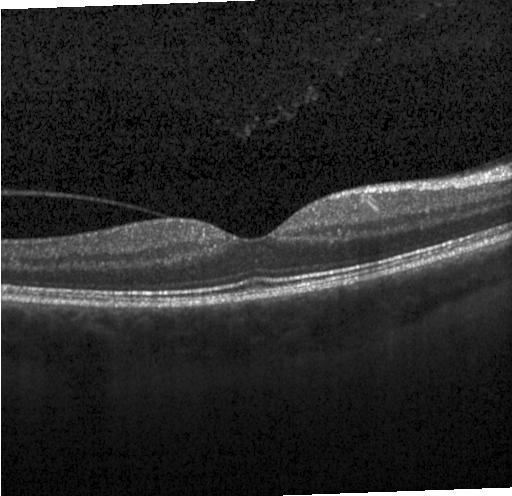
Macular scan · retinal OCT cross-section — Diagnosis: no choroidal neovascularization, diabetic macular edema, or drusen.